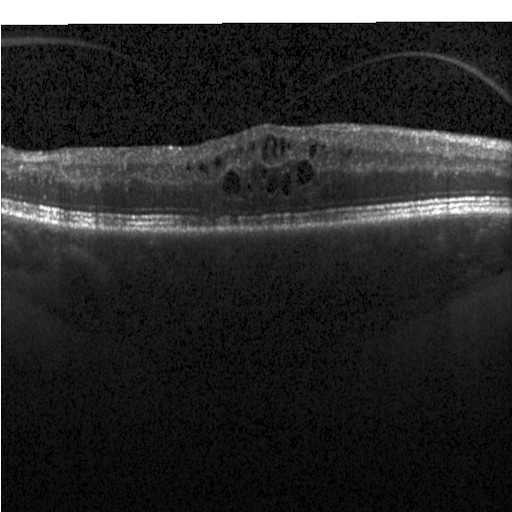 Diagnosis: diabetic macular edema (DME).